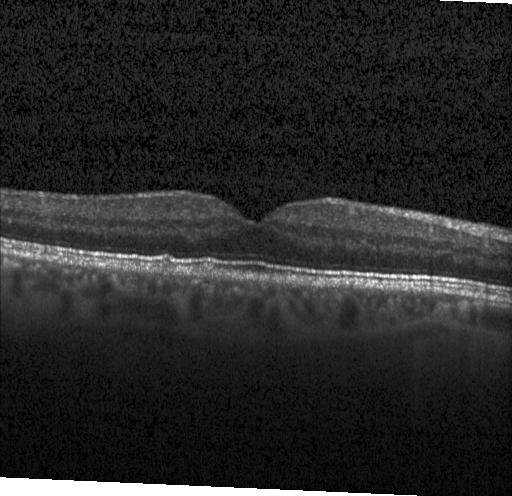

OCT B-scan showing multiple drusen.